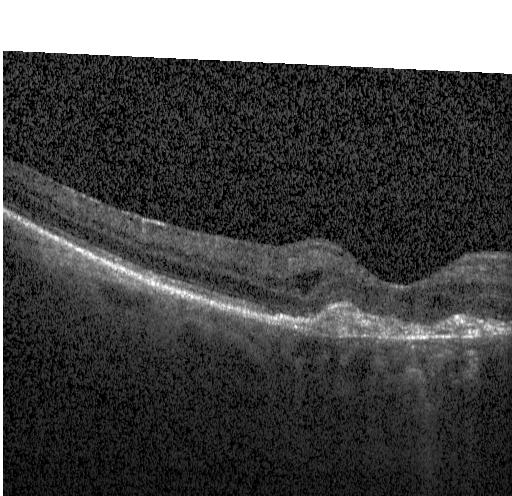
OCT finding: CNV.